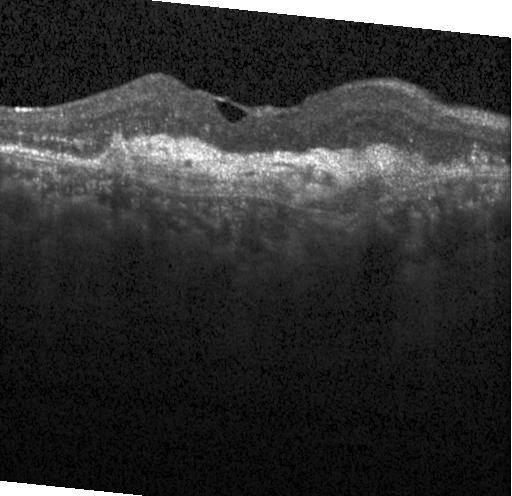
This B-scan demonstrates a choroidal neovascular membrane.